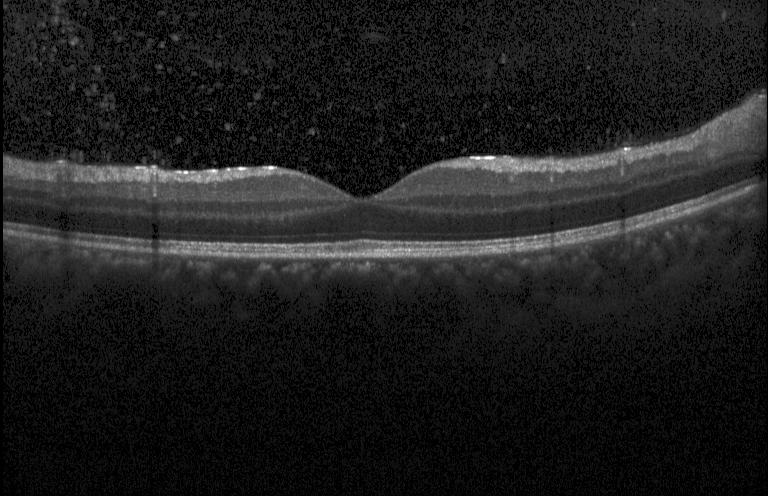

Retinal OCT cross-section. Spectral-domain OCT. Through the macula. Heidelberg Spectralis — Neither choroidal neovascularization, diabetic macular edema, nor drusen.